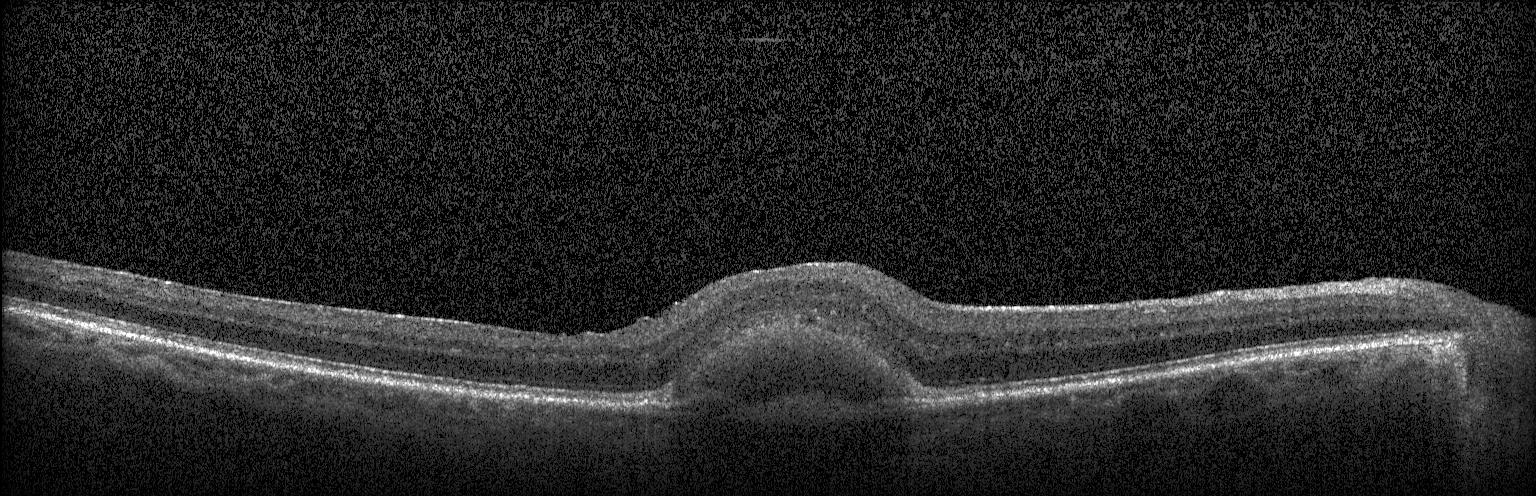
Centered on the fovea; OCT line scan.
Diagnosis: choroidal neovascularization (CNV).